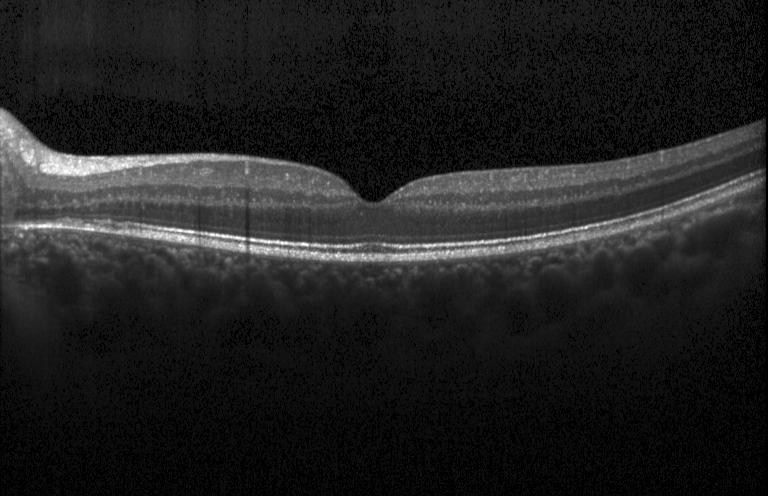 Horizontal scan through the fovea; spectral-domain optical coherence tomography; retinal OCT B-scan. Dx: neither choroidal neovascularization, diabetic macular edema, nor drusen.